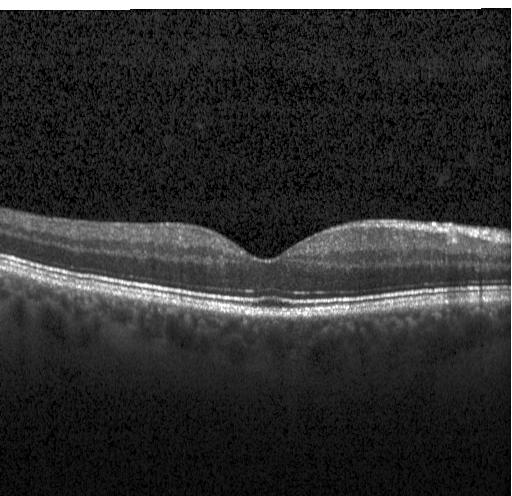
Diagnosis: no choroidal neovascularization, no diabetic macular edema, and no drusen.